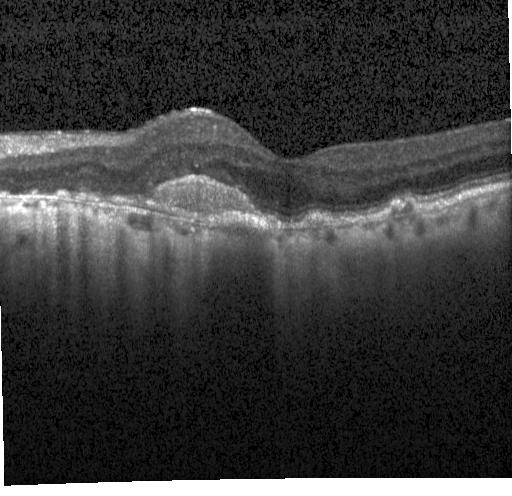

Spectral-domain OCT; retinal OCT B-scan
Impression: a choroidal neovascular membrane.